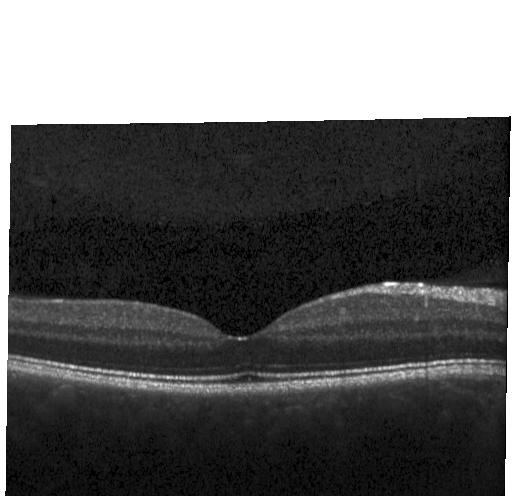

Impression: neither choroidal neovascularization, diabetic macular edema, nor drusen.